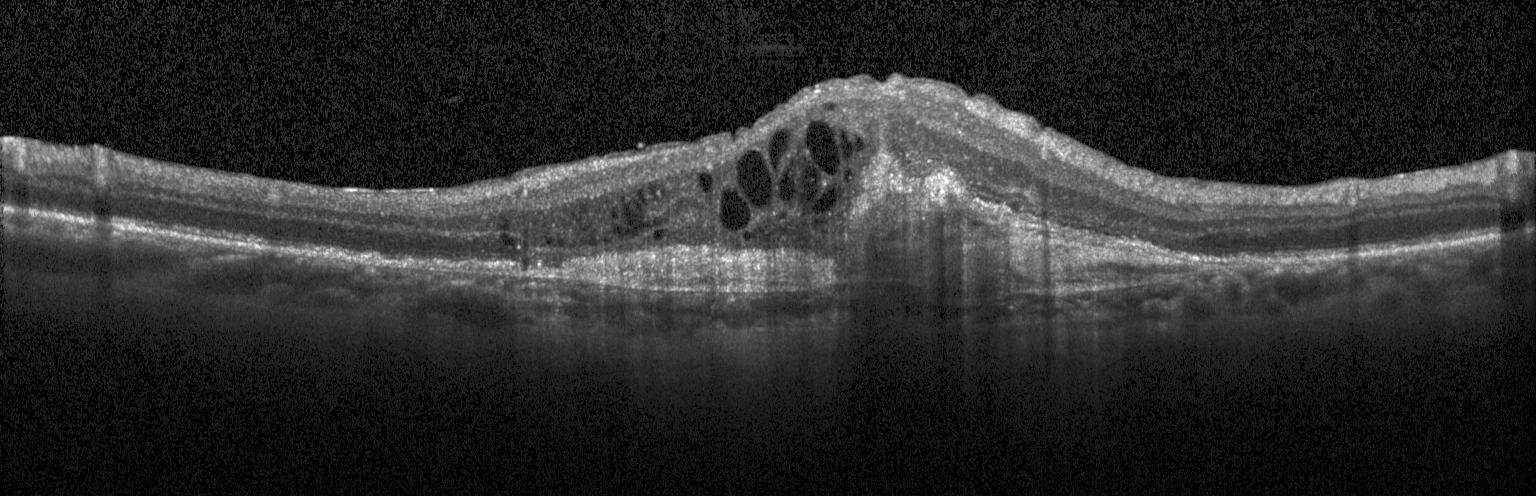
Retinal OCT cross-section
Macular OCT: choroidal neovascularization (CNV).